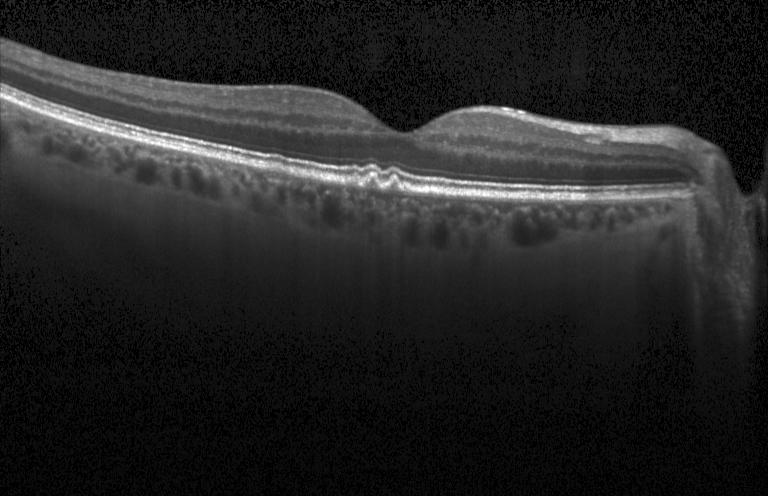

Retinal OCT B-scan
This B-scan demonstrates multiple drusen.